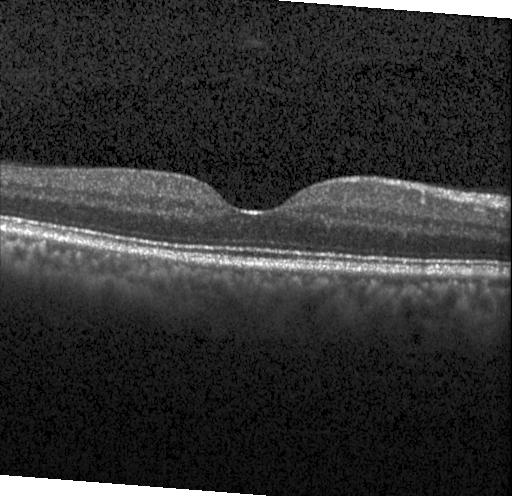 Retinal OCT B-scan. This B-scan demonstrates no choroidal neovascularization, diabetic macular edema, or drusen.